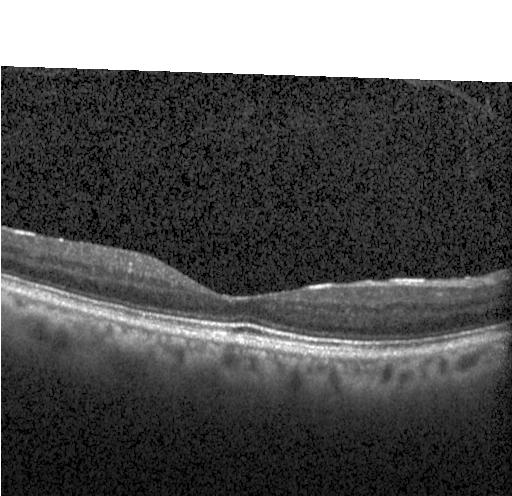 OCT B-scan showing no evidence of CNV, DME, or drusen.